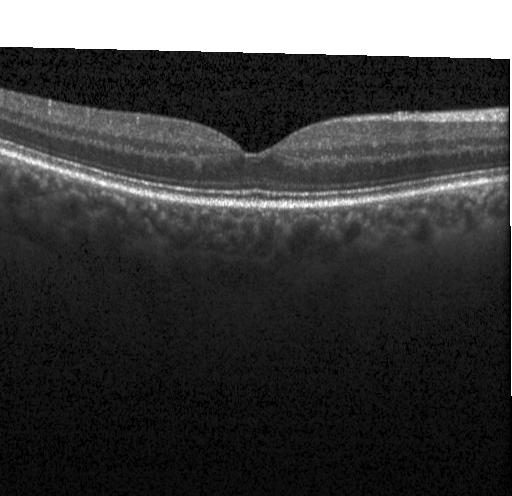 The scan shows neither choroidal neovascularization, diabetic macular edema, nor drusen.